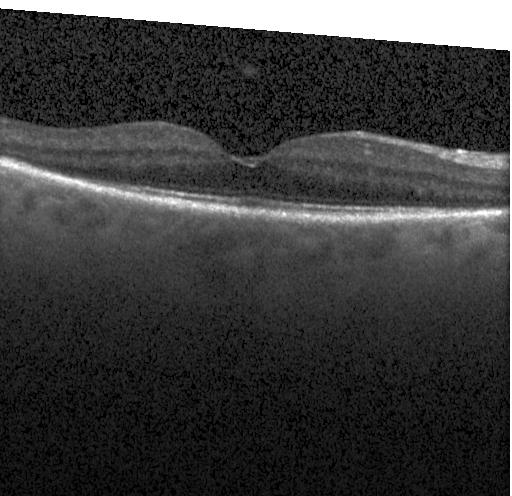 OCT B-scan; SD-OCT; centered on the fovea.
Finding: no choroidal neovascularization, diabetic macular edema, or drusen.